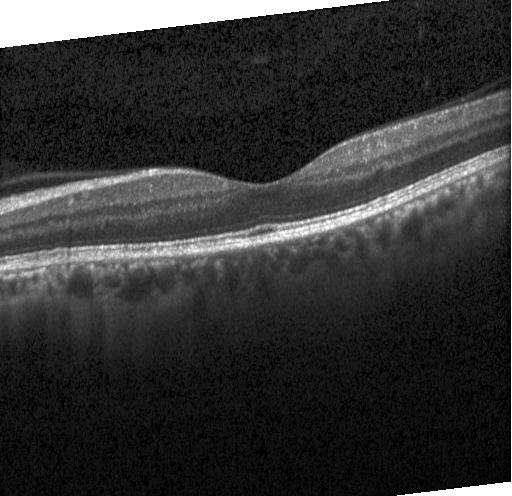

Heidelberg Spectralis, spectral-domain OCT, optical coherence tomography B-scan. Diagnosis: neither choroidal neovascularization, diabetic macular edema, nor drusen.